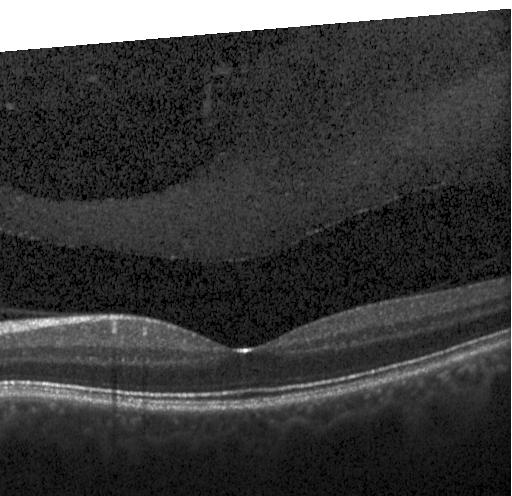

Horizontal scan through the fovea. Optical coherence tomography B-scan
The scan shows neither choroidal neovascularization, diabetic macular edema, nor drusen.